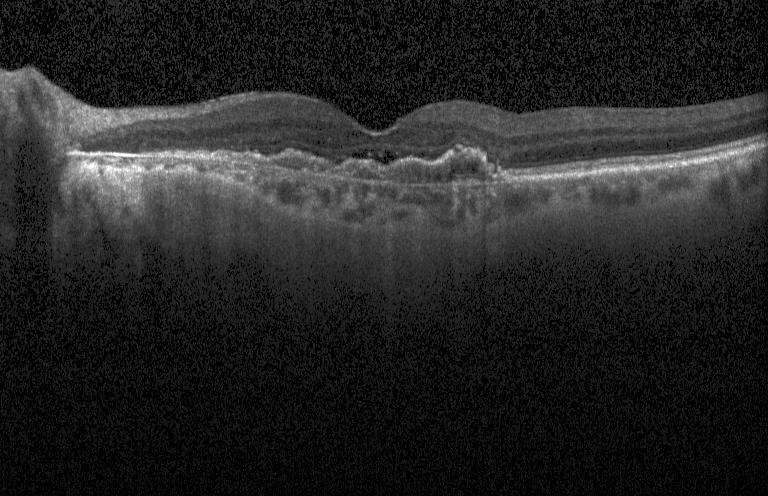 Optical coherence tomography scan; fovea-centered; acquired on a Heidelberg Spectralis. Diagnosis: a choroidal neovascular membrane.